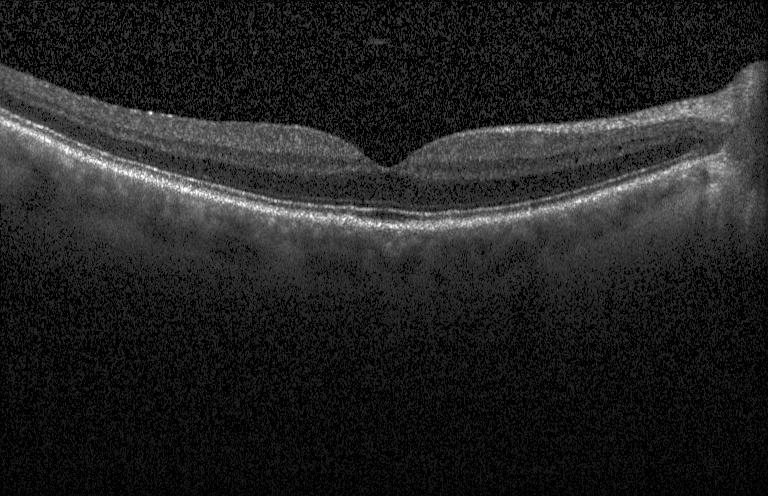 Assessment: no choroidal neovascularization, diabetic macular edema, or drusen.